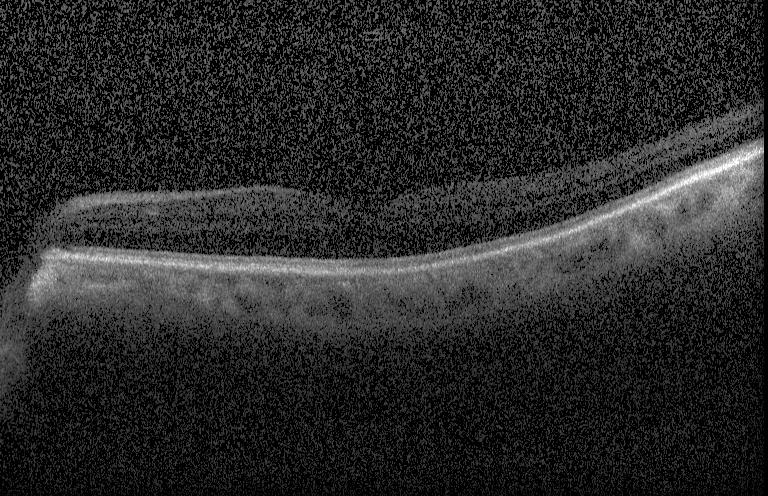
Acquired on a Heidelberg Spectralis · macular scan · SD-OCT · OCT line scan
Finding: no choroidal neovascularization, diabetic macular edema, or drusen.